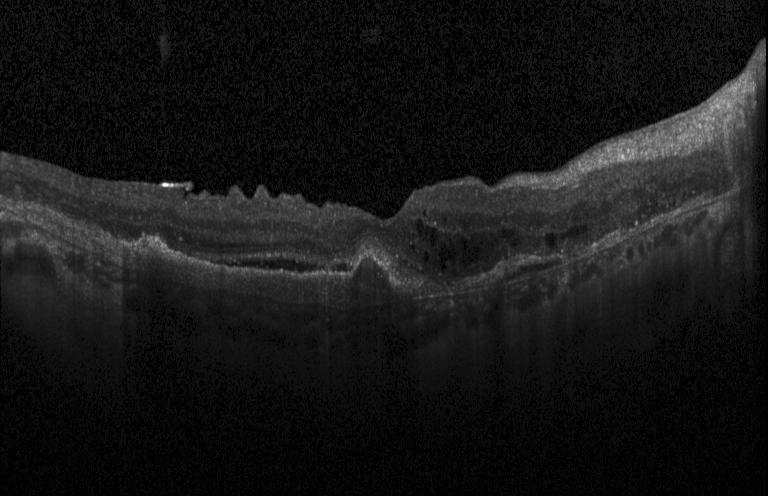
Optical coherence tomography scan, horizontal scan through the fovea, Heidelberg Spectralis, spectral-domain optical coherence tomography. Diagnosis: a choroidal neovascular membrane.